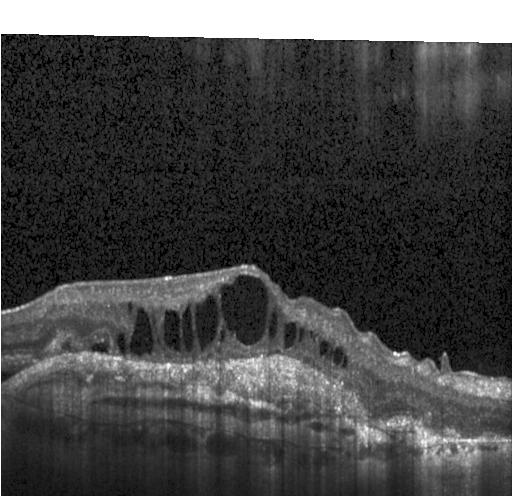 Spectral-domain OCT · optical coherence tomography B-scan — This B-scan demonstrates a choroidal neovascular membrane.